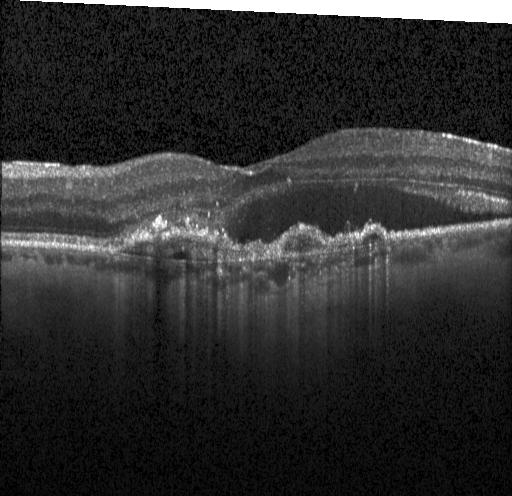 Macular OCT demonstrating a choroidal neovascular membrane.